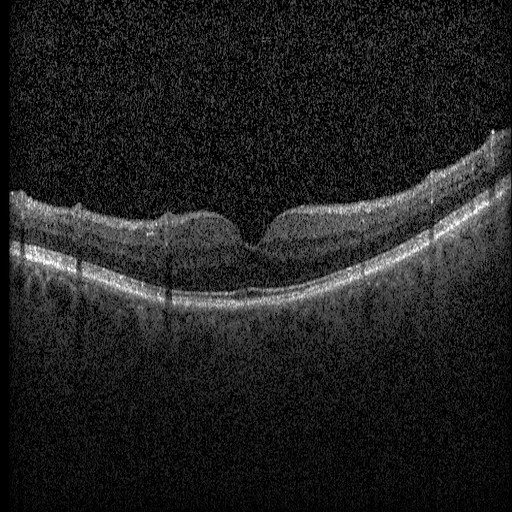

Through the macula; instrument: Heidelberg Spectralis; retinal OCT B-scan; spectral-domain optical coherence tomography. Impression: diabetic macular edema.